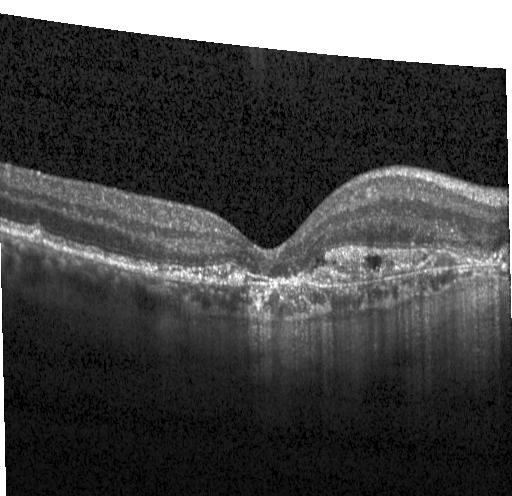 Optical coherence tomography scan · spectral-domain OCT. Dx: CNV.